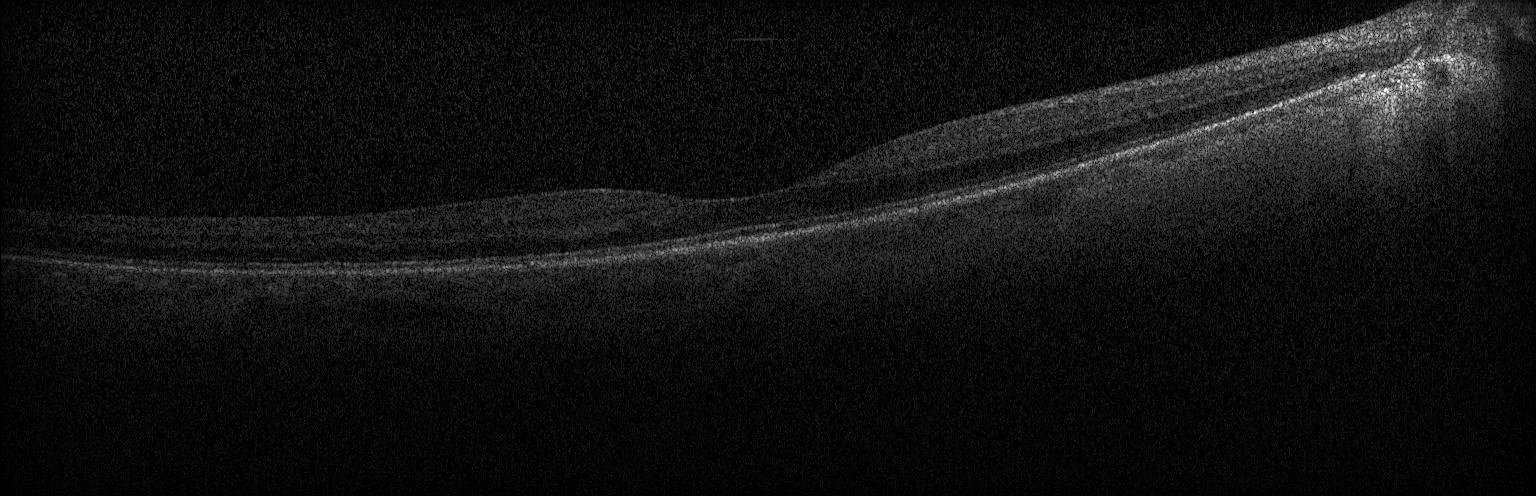 OCT line scan — Finding: no choroidal neovascularization, diabetic macular edema, or drusen.